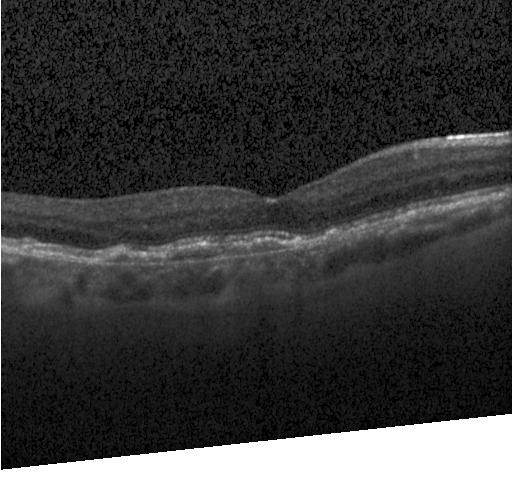 OCT line scan. Heidelberg Spectralis OCT system.
OCT finding: a choroidal neovascular membrane.